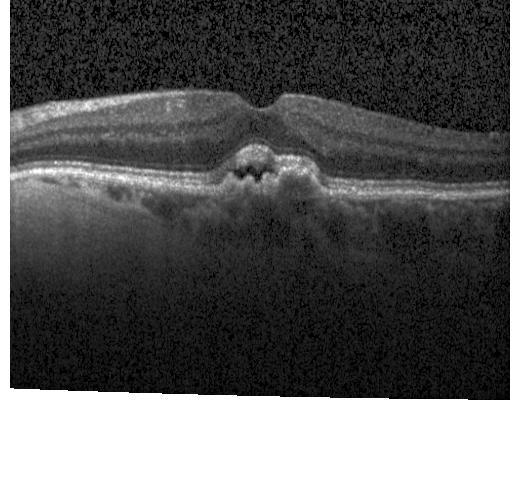

Spectral-domain optical coherence tomography · fovea-centered · retinal OCT B-scan
The scan shows CNV.